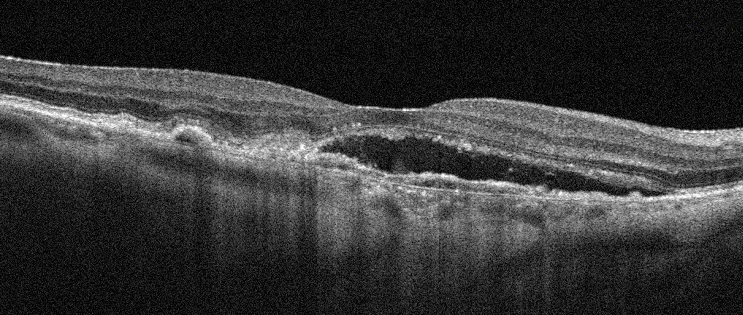

Diagnosis: age-related macular degeneration (AMD).